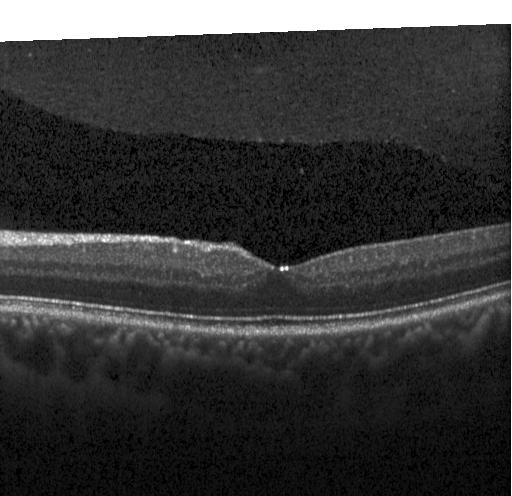
Retinal OCT B-scan. This B-scan demonstrates no CNV, no DME, and no drusen.